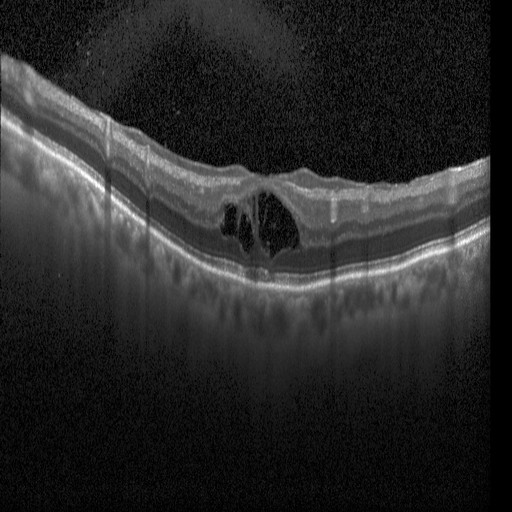 Fovea-centered, OCT line scan — This B-scan demonstrates DME.